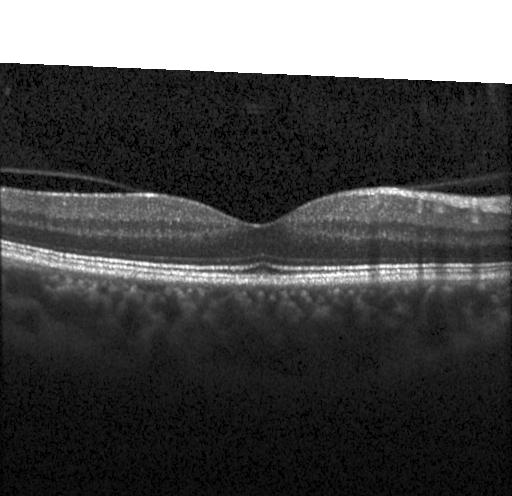 This B-scan demonstrates no evidence of choroidal neovascularization, diabetic macular edema, or drusen.